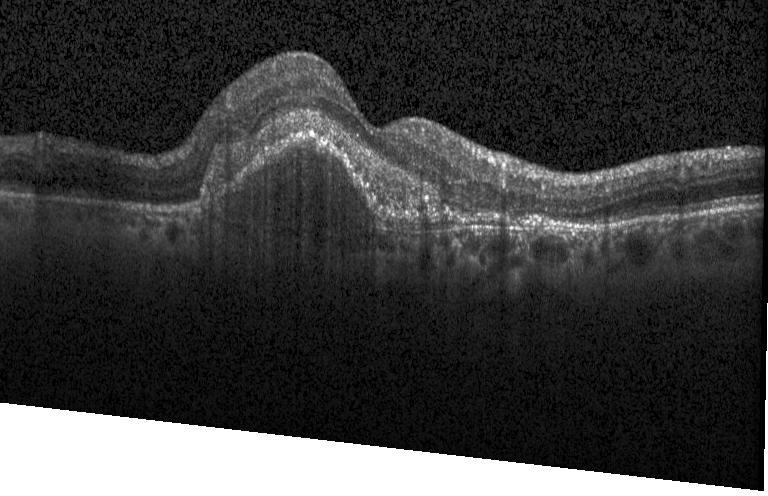
OCT B-scan · spectral-domain optical coherence tomography. The scan shows a choroidal neovascular membrane.